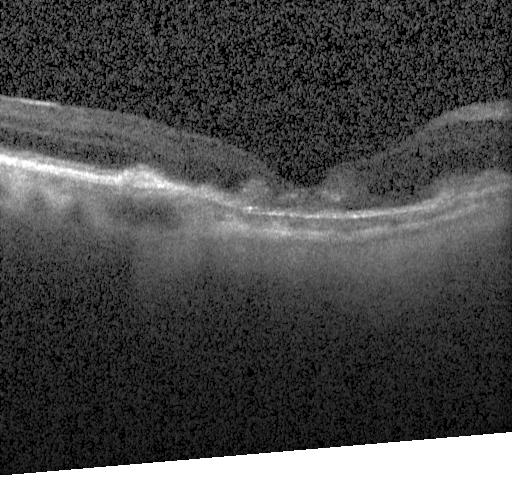
Horizontal scan through the fovea, Heidelberg Spectralis OCT system, optical coherence tomography B-scan — Macular OCT: choroidal neovascularization (CNV).